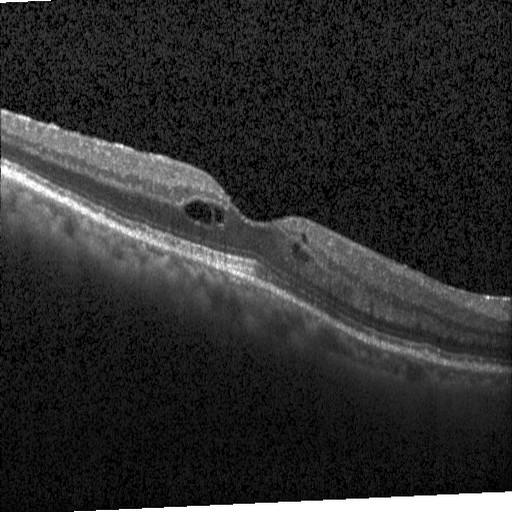

The scan shows DME.